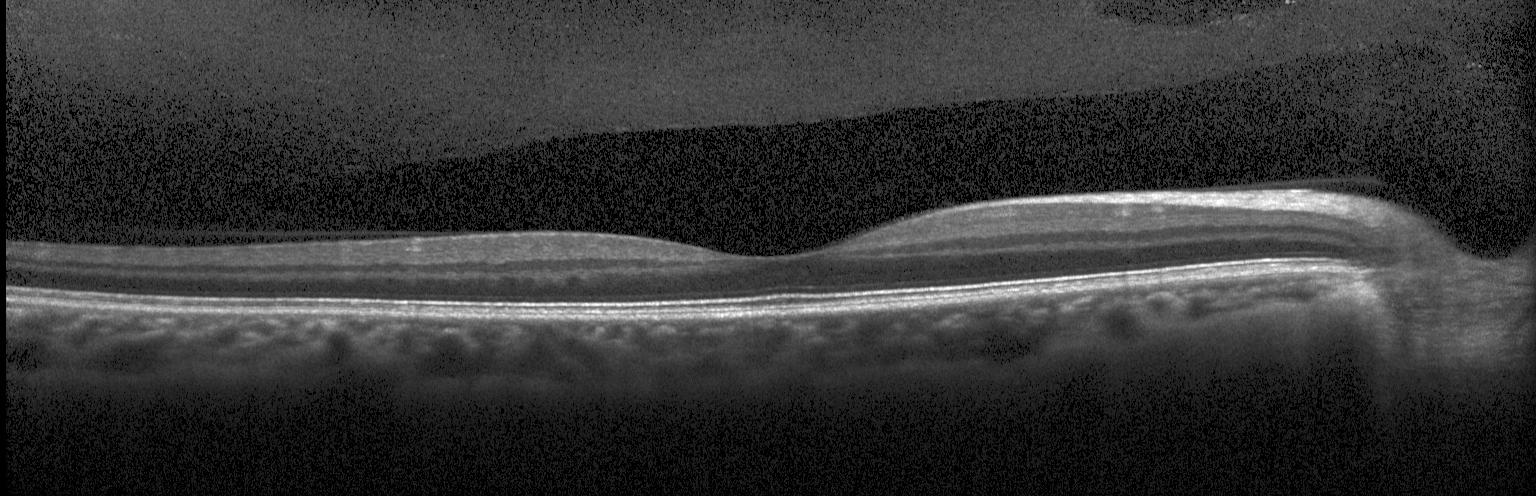

OCT line scan — This B-scan demonstrates no evidence of choroidal neovascularization, diabetic macular edema, or drusen.